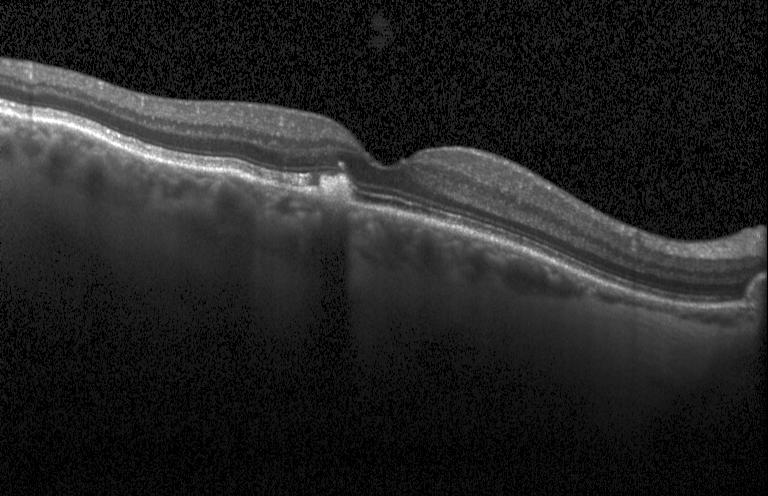 Diagnosis: sub-RPE drusenoid deposits.